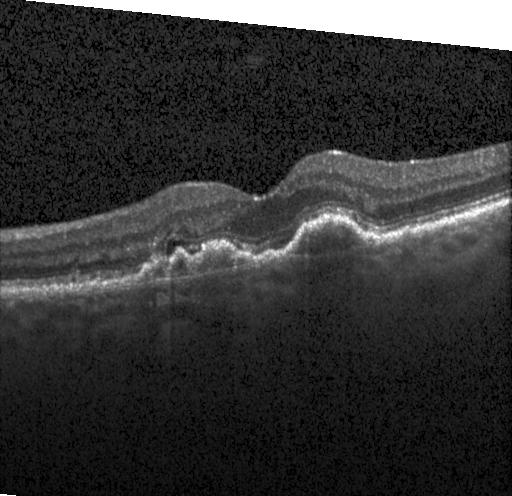 Diagnosis: a choroidal neovascular membrane.